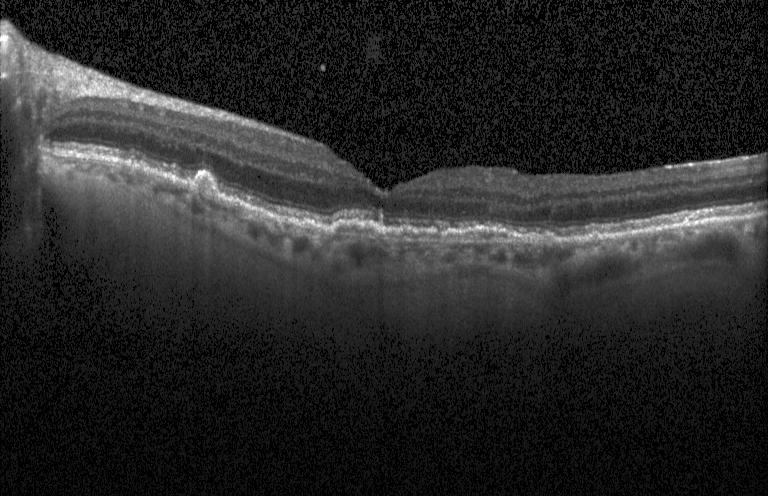 OCT B-scan showing sub-RPE drusenoid deposits.